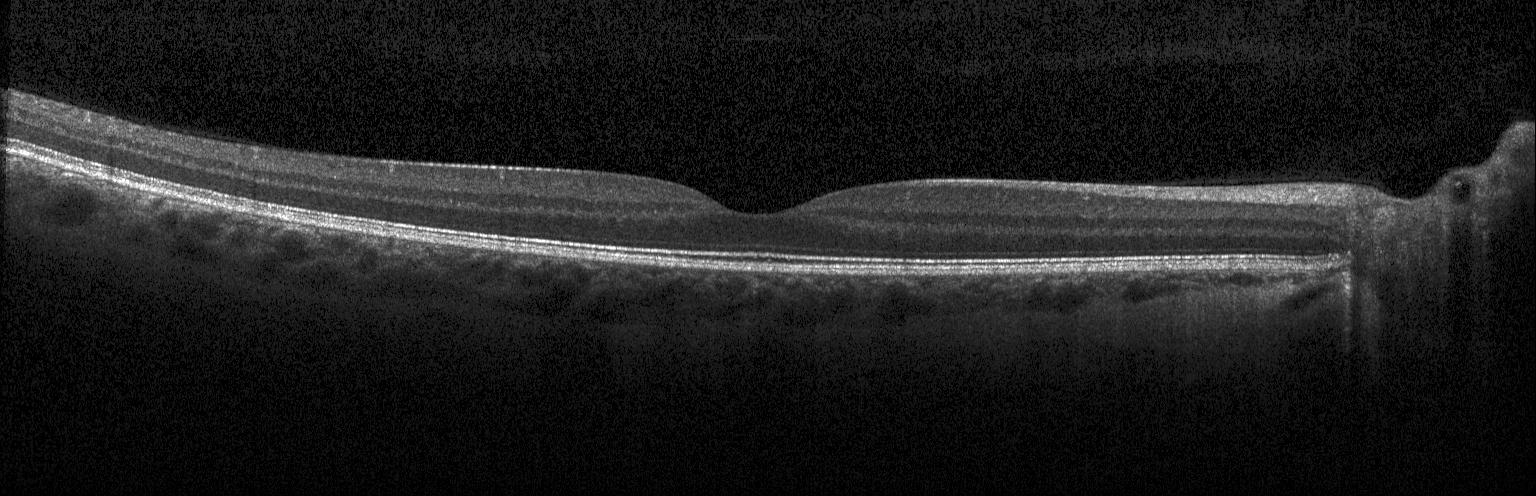 Spectral-domain optical coherence tomography. Heidelberg Spectralis OCT system. Horizontal scan through the fovea. Optical coherence tomography scan.
Macular OCT: neither choroidal neovascularization, diabetic macular edema, nor drusen.